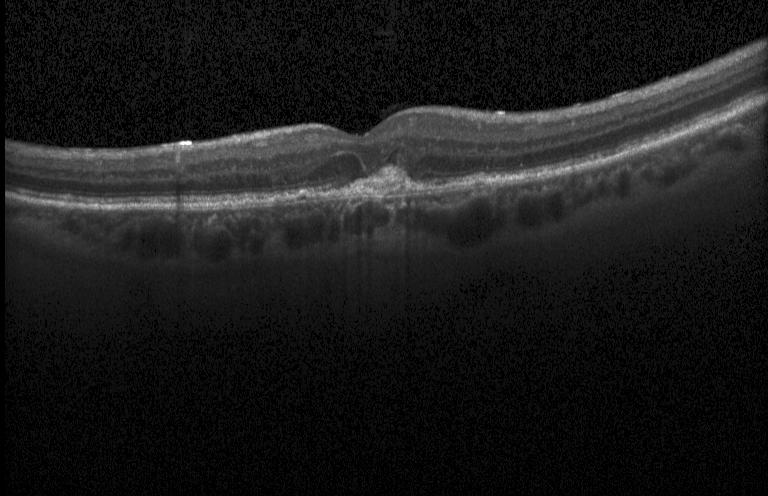

Horizontal scan through the fovea. Spectral-domain optical coherence tomography. Acquired on a Heidelberg Spectralis. Retinal OCT B-scan. This B-scan demonstrates choroidal neovascularization.